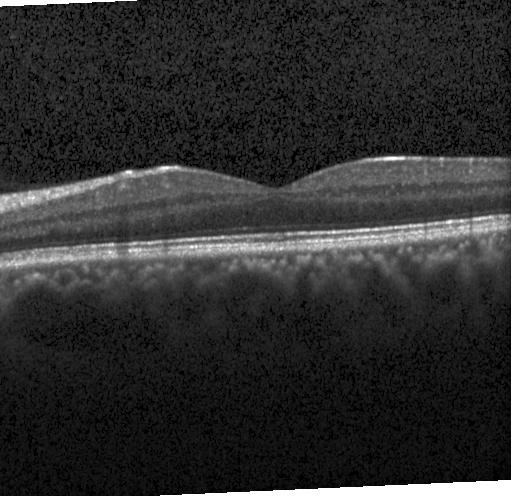 Retinal OCT cross-section. Assessment: neither choroidal neovascularization, diabetic macular edema, nor drusen.